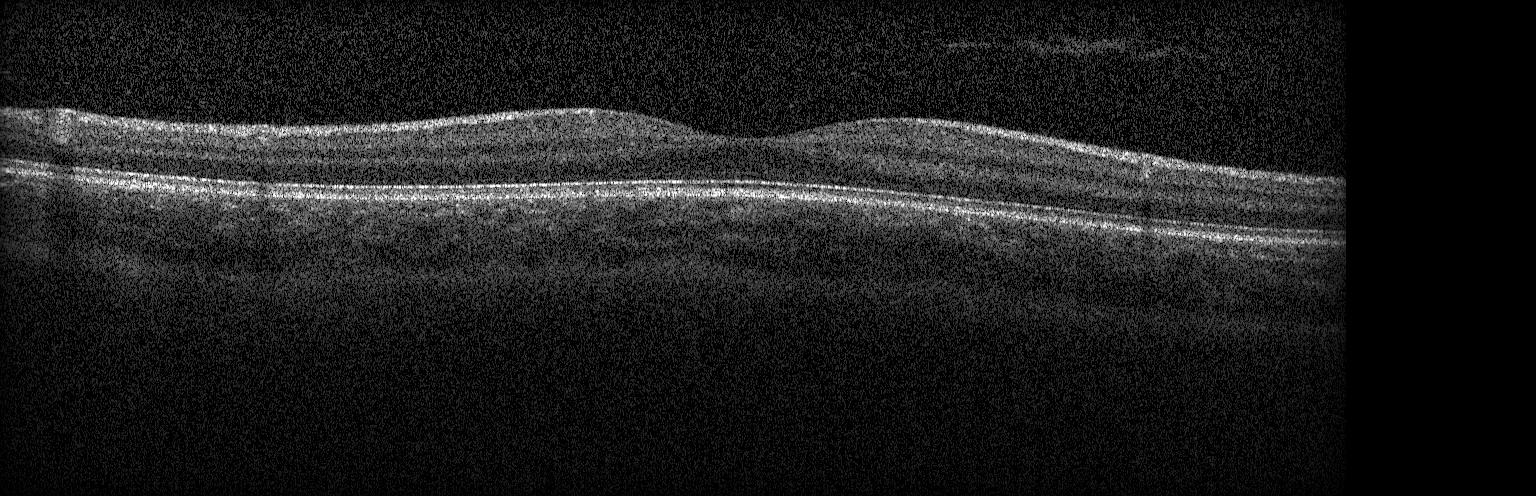
Retinal OCT cross-section showing no choroidal neovascularization, diabetic macular edema, or drusen.